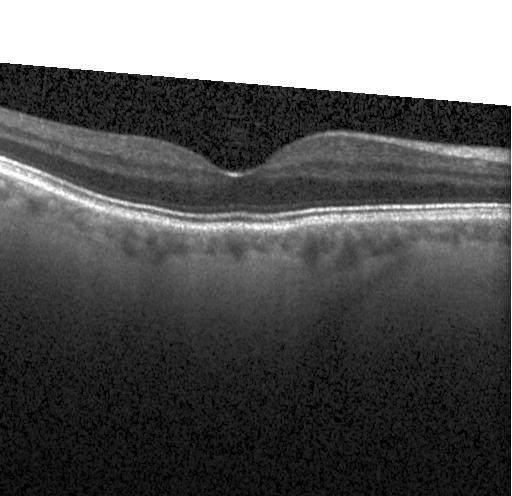

OCT line scan. Macular OCT: no CNV, DME, or drusen.